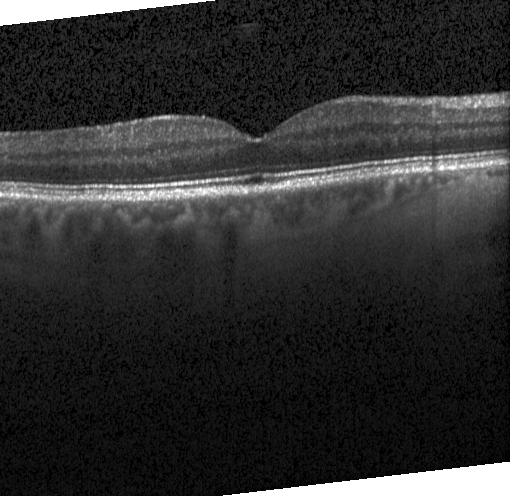 Optical coherence tomography B-scan
The scan shows no CNV, DME, or drusen.